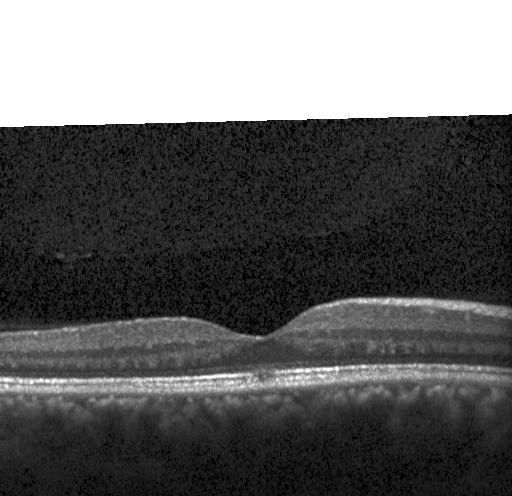

Retinal OCT cross-section · acquired on a Heidelberg Spectralis · macular scan · SD-OCT. Finding: no CNV, DME, or drusen.